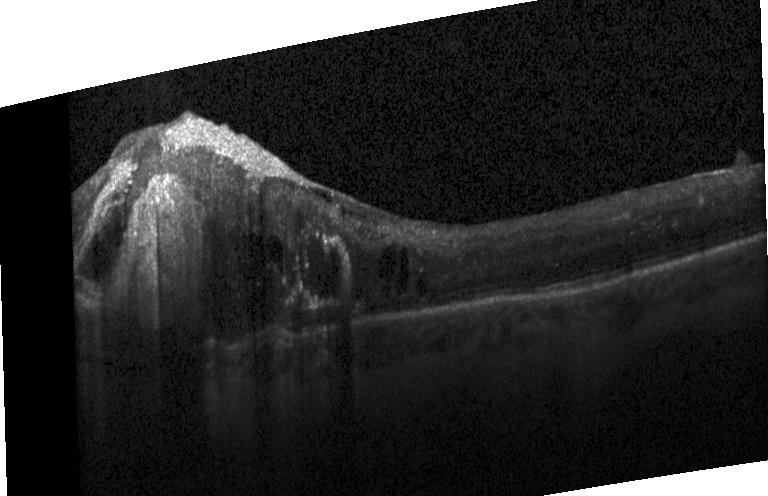

This B-scan demonstrates a choroidal neovascular membrane.